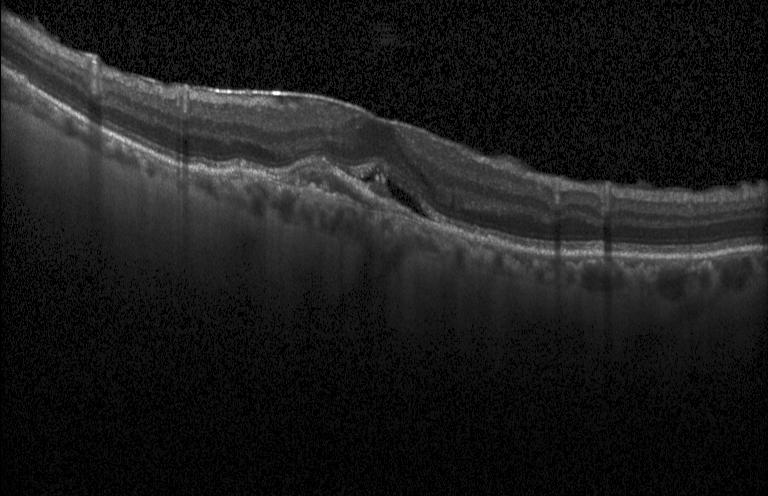 Centered on the fovea, retinal OCT B-scan, spectral-domain OCT, acquired on a Heidelberg Spectralis — The scan shows a choroidal neovascular membrane.